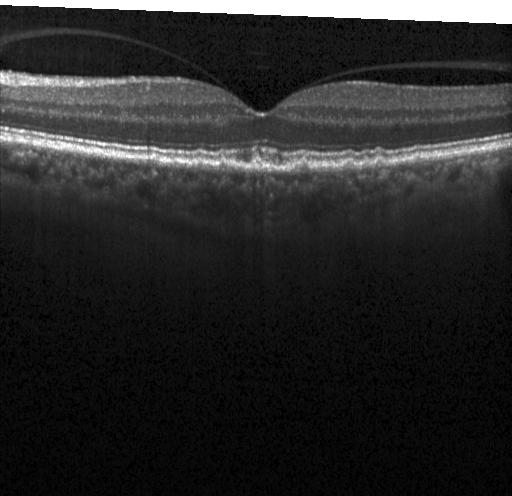

Dx: sub-RPE drusenoid deposits.